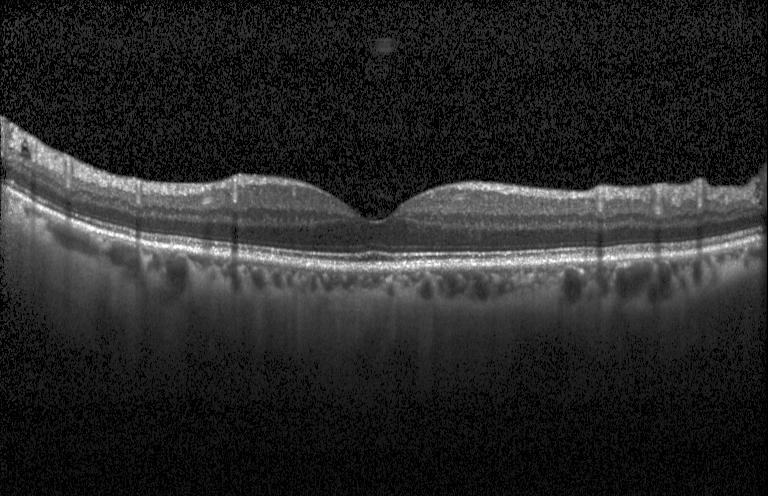
Optical coherence tomography scan. Diagnosis: no CNV, DME, or drusen.